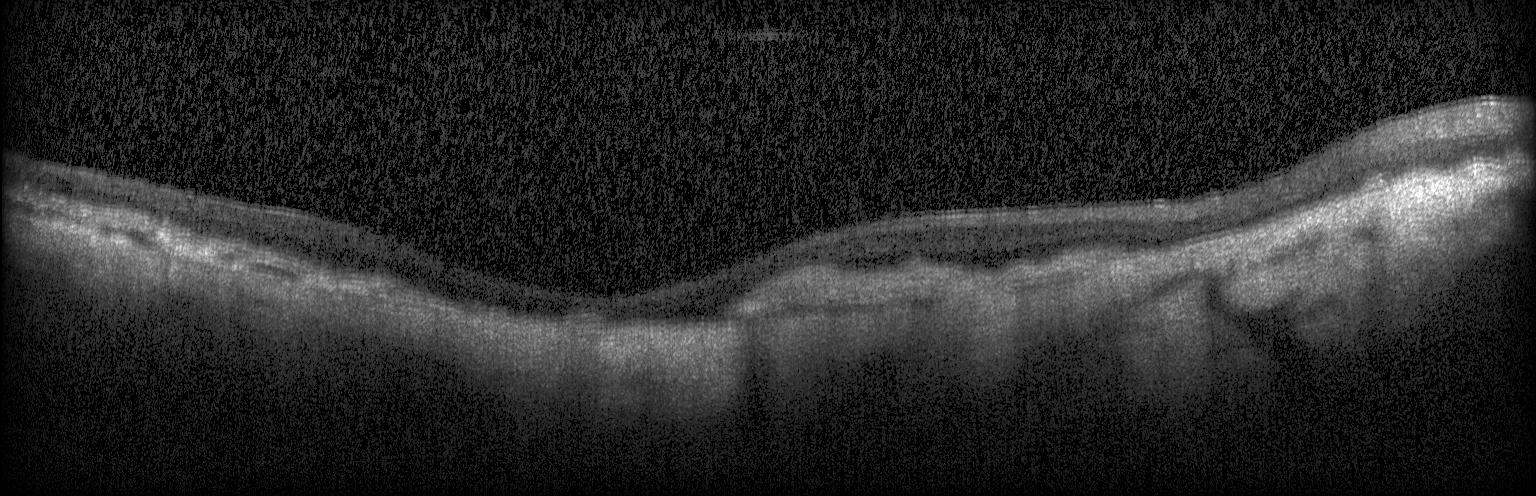
Spectral-domain optical coherence tomography, macular scan, retinal OCT cross-section — Assessment: a choroidal neovascular membrane.